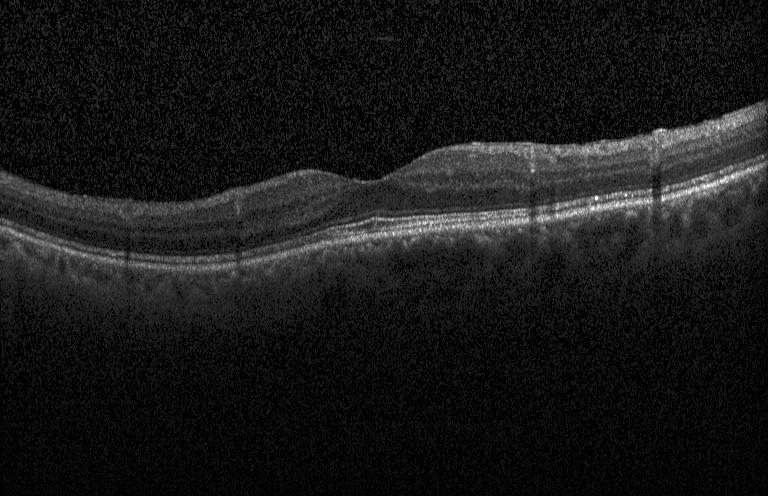

OCT B-scan · acquired on a Heidelberg Spectralis · through the macula · spectral-domain optical coherence tomography
Finding: no choroidal neovascularization, diabetic macular edema, or drusen.